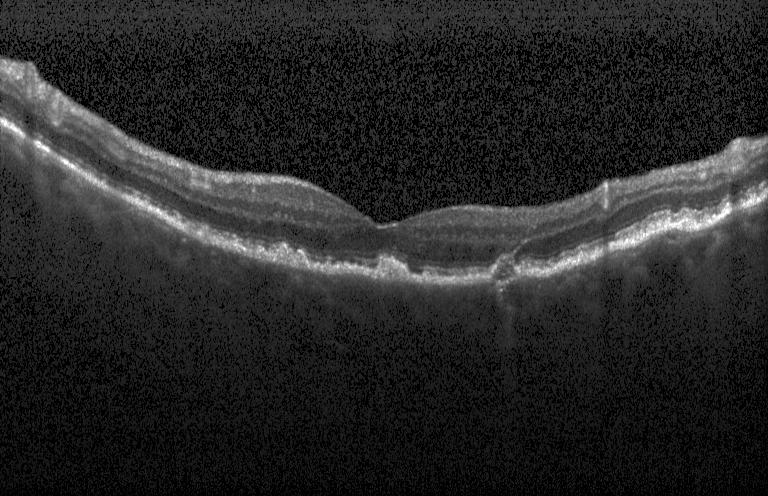
Heidelberg Spectralis OCT system. Spectral-domain optical coherence tomography. Retinal OCT cross-section. Horizontal scan through the fovea — Diagnosis: choroidal neovascularization (CNV).